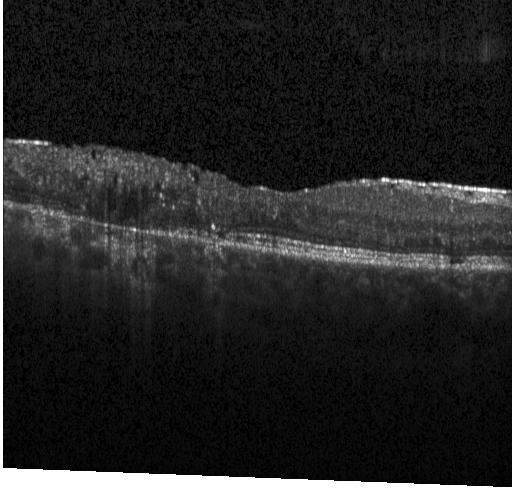 Spectral-domain OCT B-scan: diabetic macular edema.